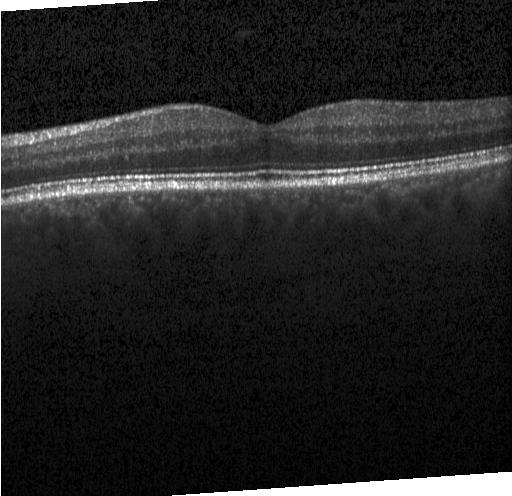 Retinal OCT cross-section; instrument: Heidelberg Spectralis; SD-OCT — This B-scan demonstrates neither CNV, DME, nor drusen.